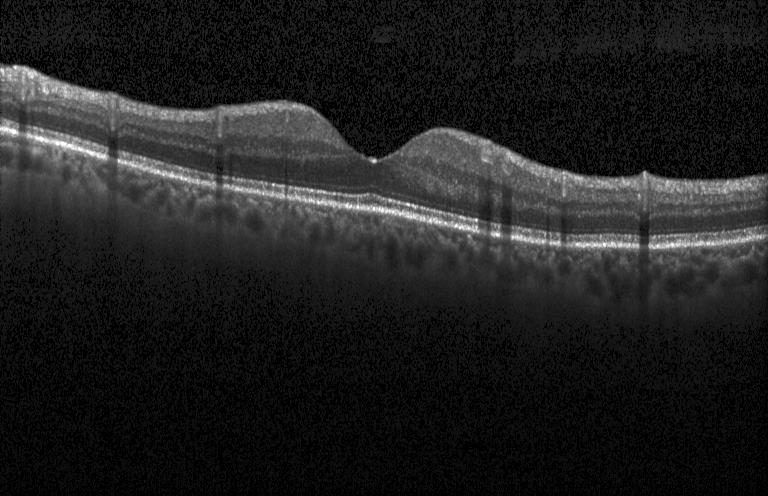
Retinal OCT B-scan — Impression: no CNV, DME, or drusen.